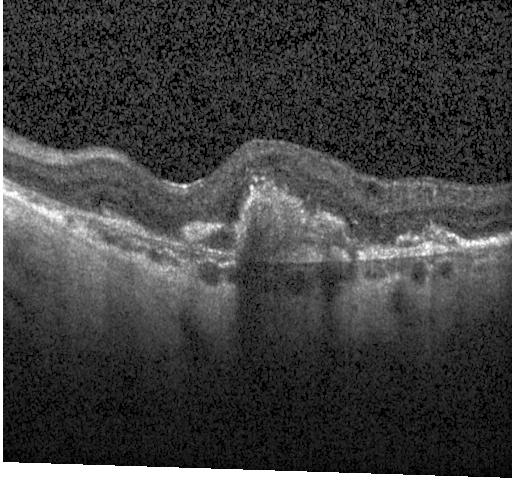
OCT B-scan, fovea-centered, spectral-domain OCT.
Dx: choroidal neovascularization.